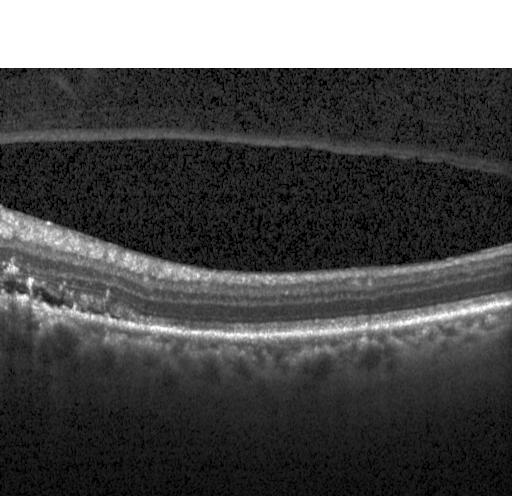

SD-OCT, retinal OCT cross-section — Diagnosis: CNV.